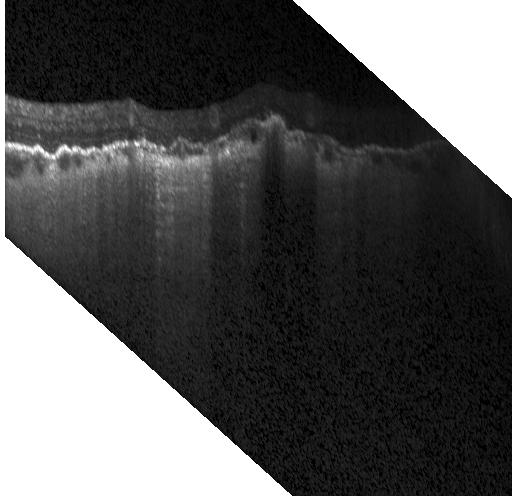 Retinal OCT B-scan.
Impression: CNV.